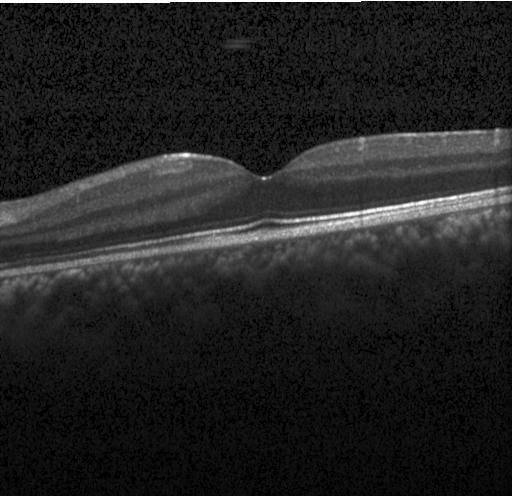
Dx: no choroidal neovascularization, no diabetic macular edema, and no drusen.